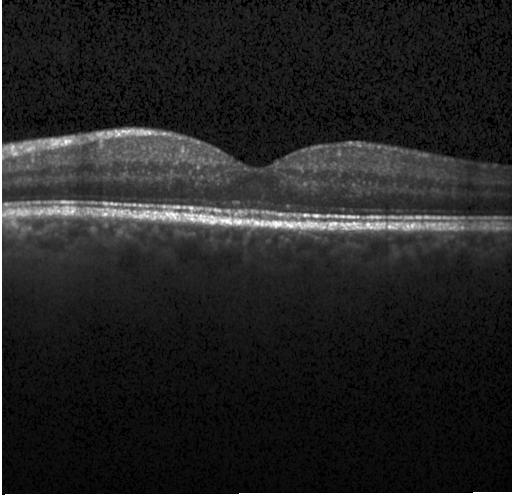

Acquired on a Heidelberg Spectralis. OCT B-scan. Dx: no choroidal neovascularization, no diabetic macular edema, and no drusen.